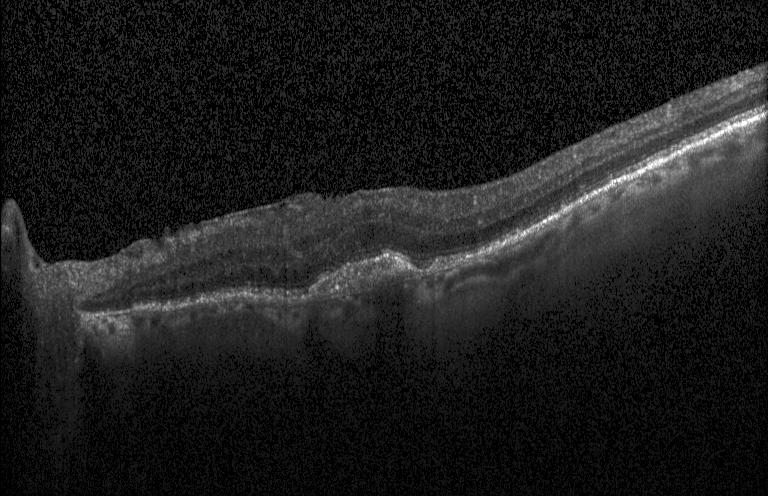
OCT line scan
Diagnosis: a choroidal neovascular membrane.